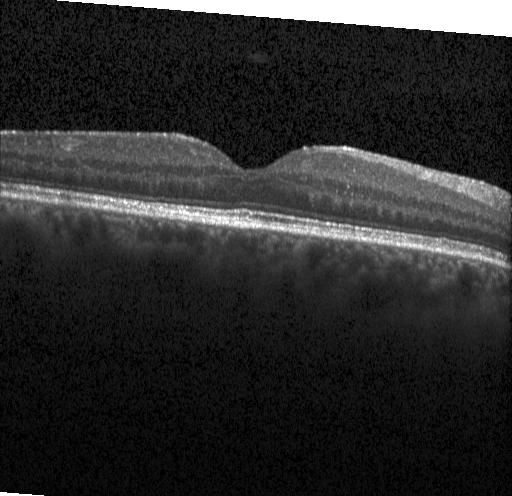
Assessment: neither choroidal neovascularization, diabetic macular edema, nor drusen.